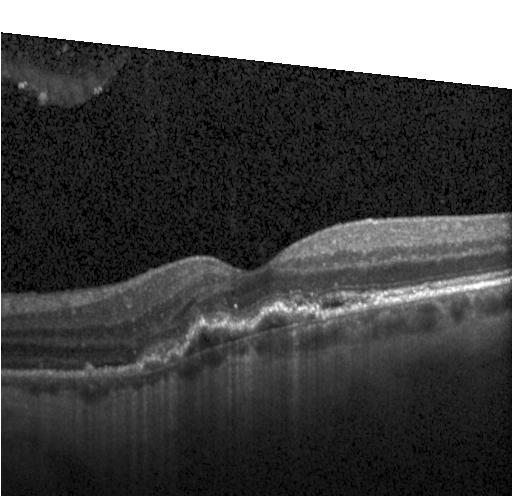
Spectral-domain OCT B-scan: CNV.